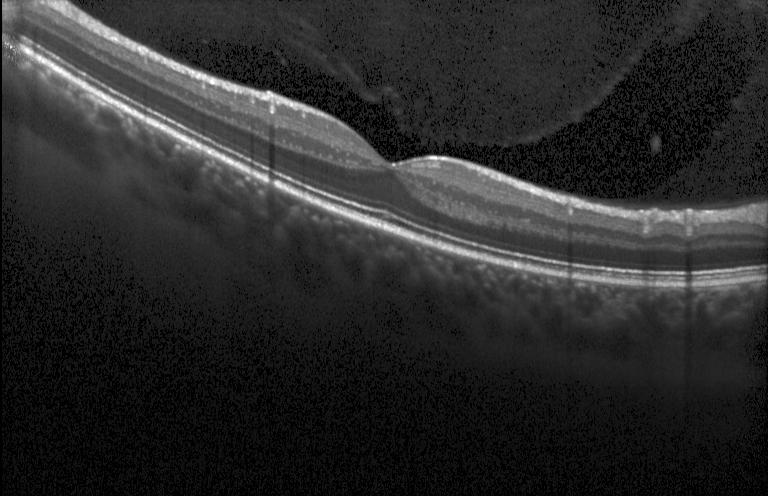

OCT scan showing no choroidal neovascularization, diabetic macular edema, or drusen.